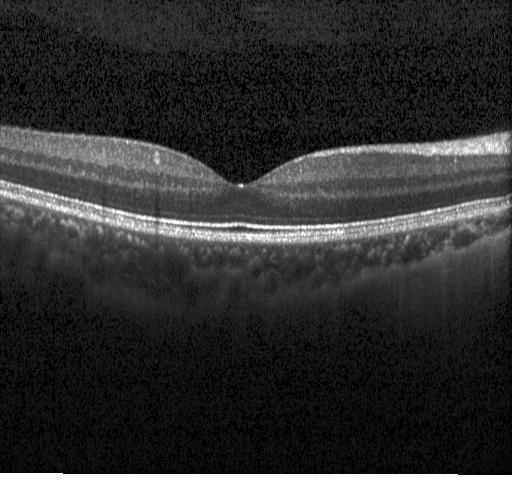
Horizontal scan through the fovea, spectral-domain OCT, retinal OCT cross-section. The scan shows no choroidal neovascularization, no diabetic macular edema, and no drusen.